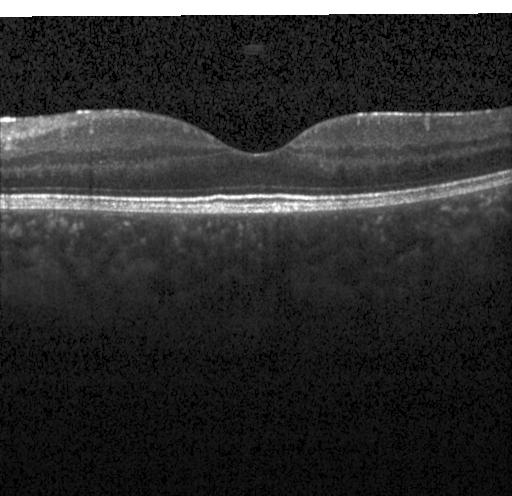
Acquired on a Heidelberg Spectralis. Retinal OCT B-scan. SD-OCT. Centered on the fovea.
Dx: no CNV, DME, or drusen.